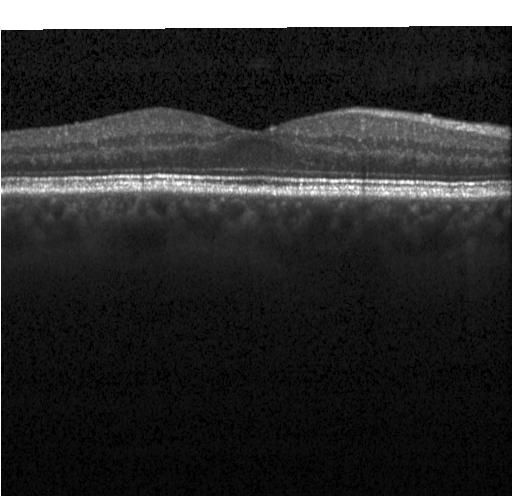
Retinal OCT cross-section showing neither CNV, DME, nor drusen.